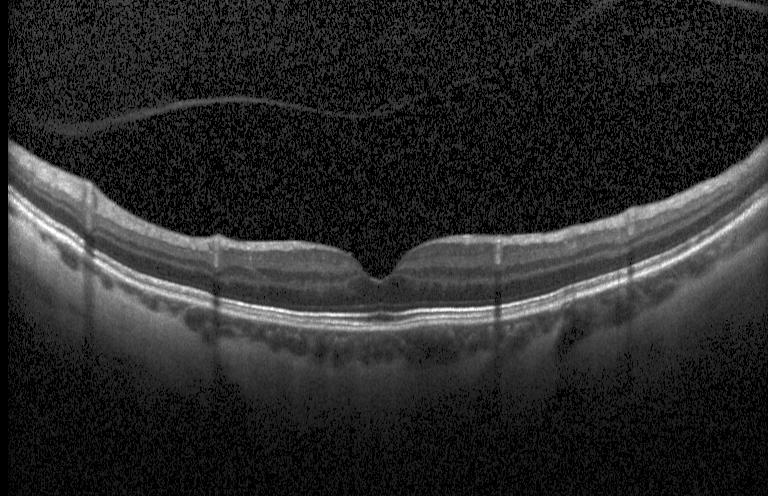

Diagnosis: no choroidal neovascularization, diabetic macular edema, or drusen.